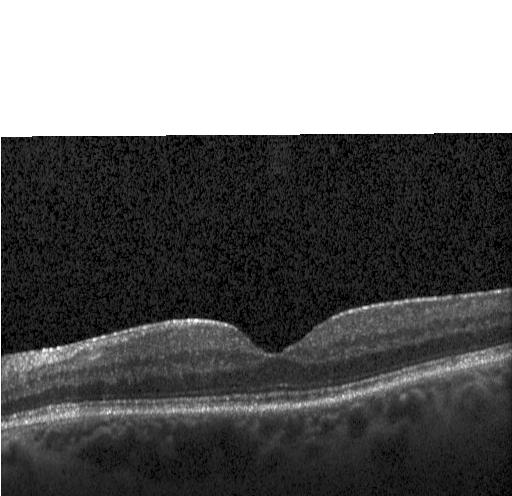 Optical coherence tomography scan · fovea-centered
This B-scan demonstrates no choroidal neovascularization, diabetic macular edema, or drusen.